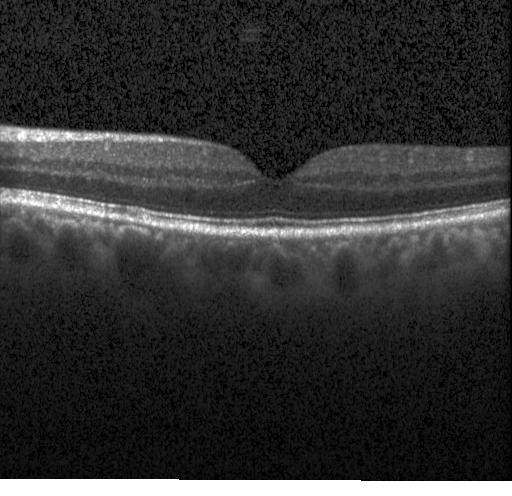 Optical coherence tomography B-scan; centered on the fovea.
The scan shows no choroidal neovascularization, diabetic macular edema, or drusen.